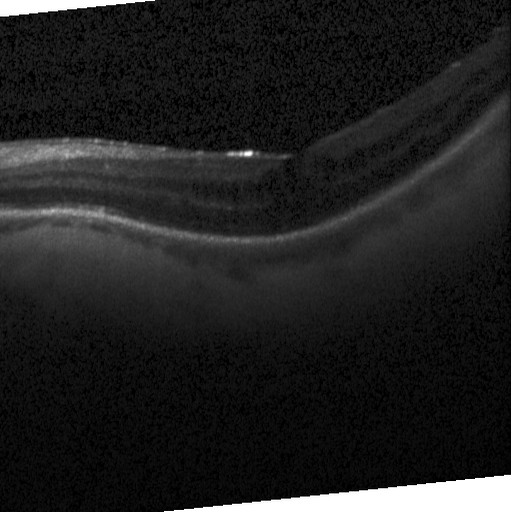

Diagnosis: DME.